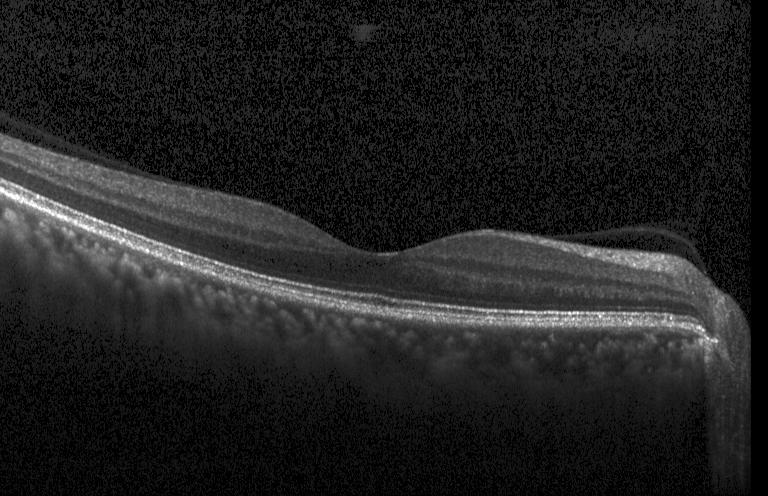

OCT B-scan, fovea-centered, spectral-domain OCT
This B-scan demonstrates no evidence of choroidal neovascularization, diabetic macular edema, or drusen.